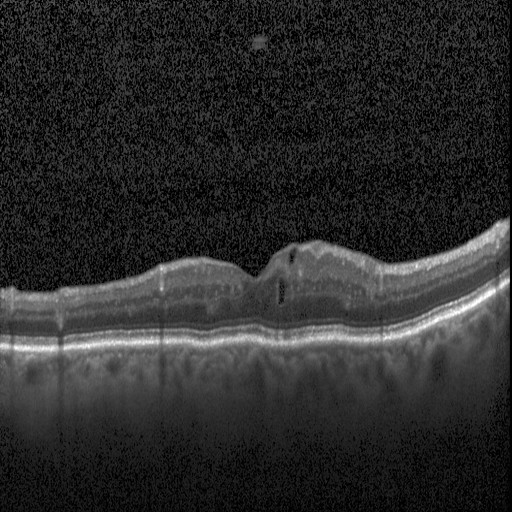
Heidelberg Spectralis; spectral-domain OCT; OCT B-scan; fovea-centered.
Diabetic macular edema.